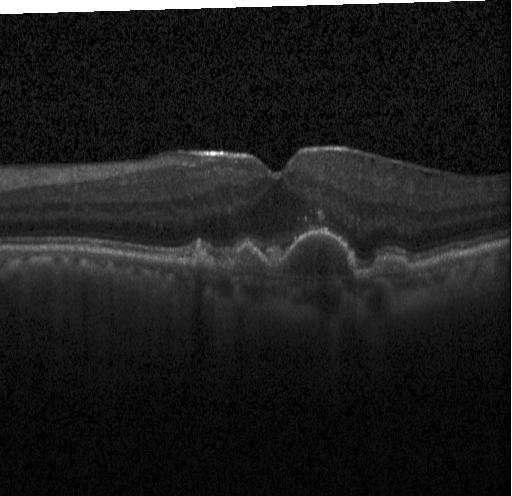
Retinal OCT B-scan
Impression: choroidal neovascularization (CNV).